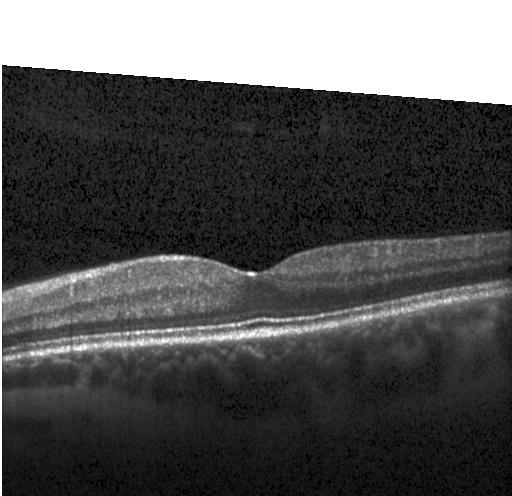 Heidelberg Spectralis OCT system; spectral-domain OCT; through the macula; optical coherence tomography scan. Finding: no CNV, no DME, and no drusen.